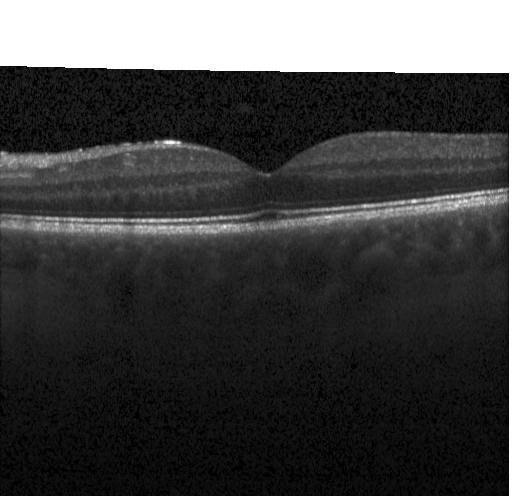

Optical coherence tomography B-scan · centered on the fovea.
Finding: neither CNV, DME, nor drusen.